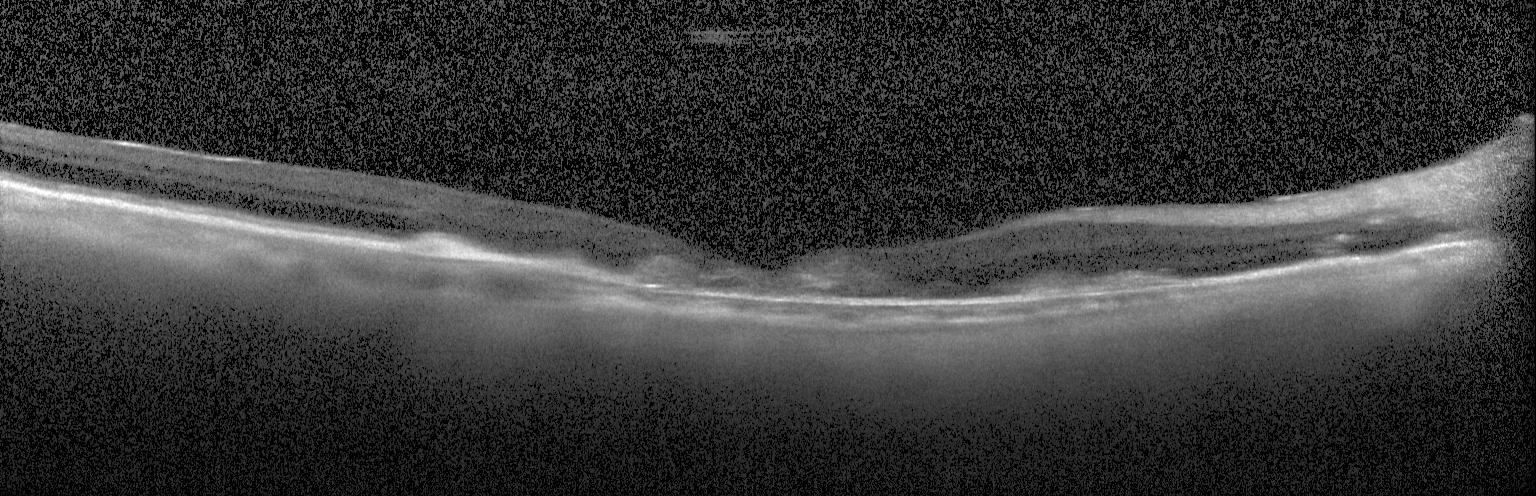
The scan shows choroidal neovascularization (CNV).